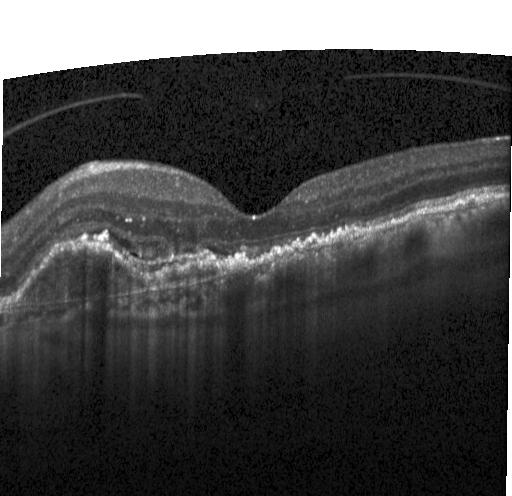

Retinal OCT cross-section showing a choroidal neovascular membrane.